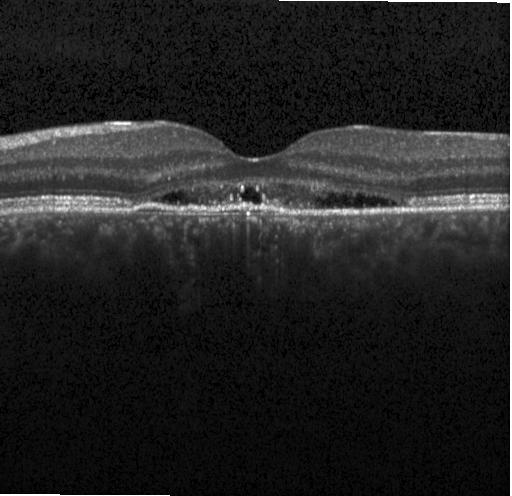

Spectral-domain OCT B-scan: choroidal neovascularization.